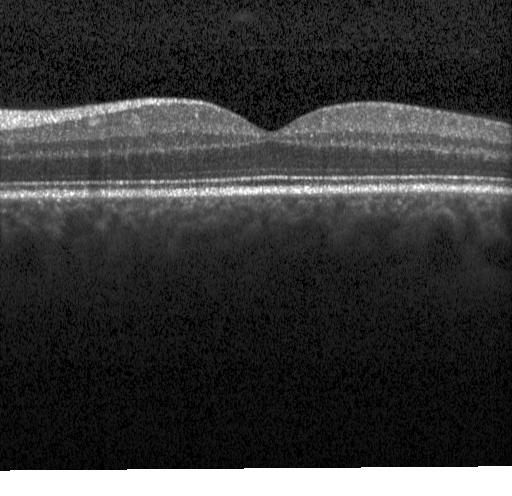 SD-OCT; macular scan; instrument: Heidelberg Spectralis; retinal OCT cross-section — Dx: no choroidal neovascularization, no diabetic macular edema, and no drusen.